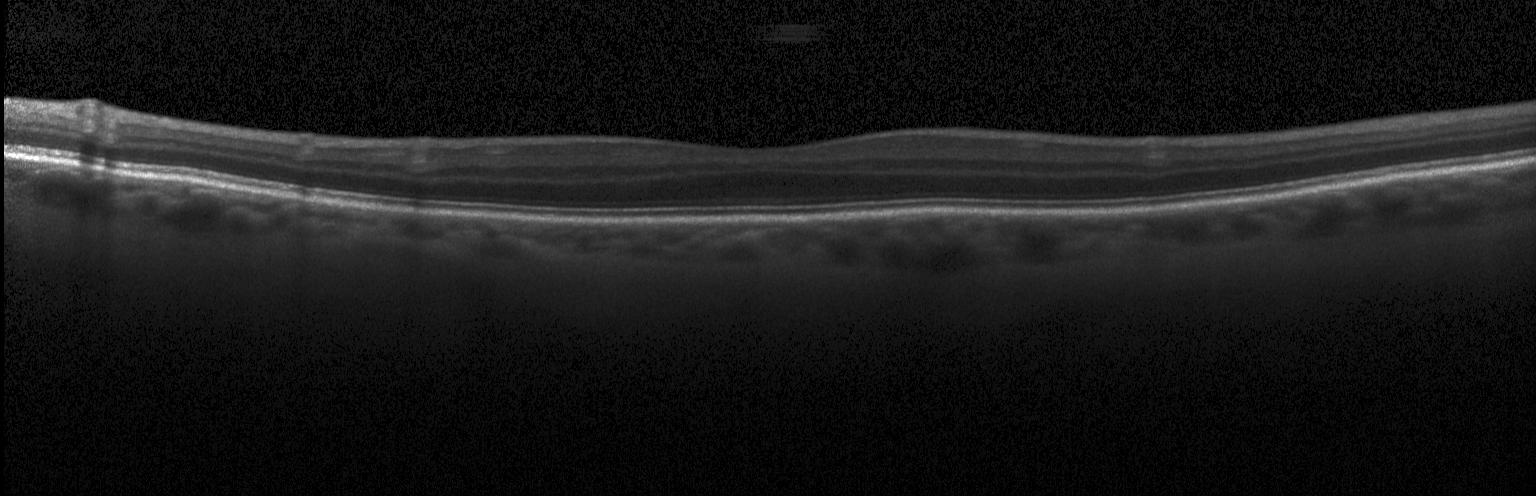

OCT finding: no choroidal neovascularization, diabetic macular edema, or drusen.